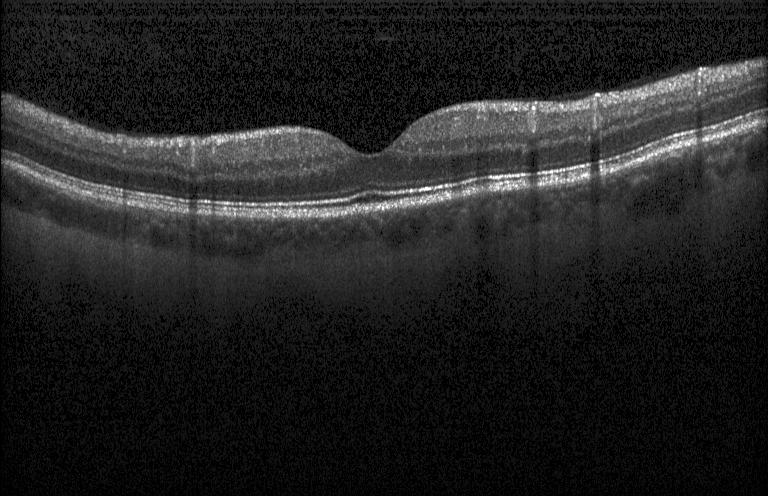

Optical coherence tomography scan, instrument: Heidelberg Spectralis, SD-OCT
Macular OCT: no choroidal neovascularization, no diabetic macular edema, and no drusen.